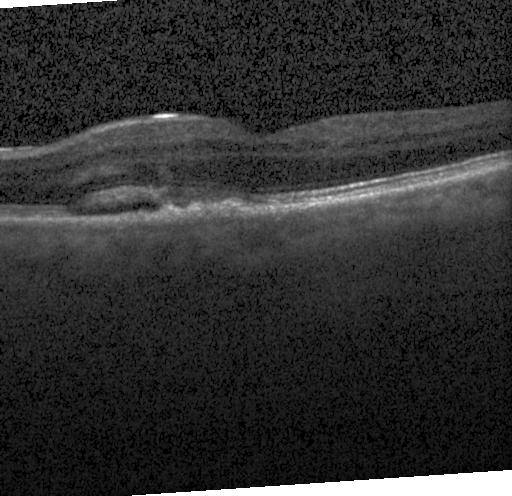
Optical coherence tomography B-scan; centered on the fovea — Finding: a choroidal neovascular membrane.